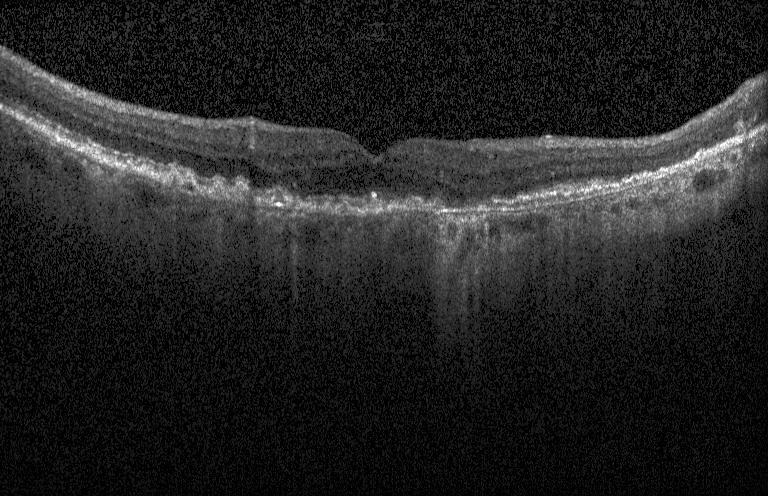 OCT B-scan, horizontal scan through the fovea, acquired on a Heidelberg Spectralis — The scan shows a choroidal neovascular membrane.